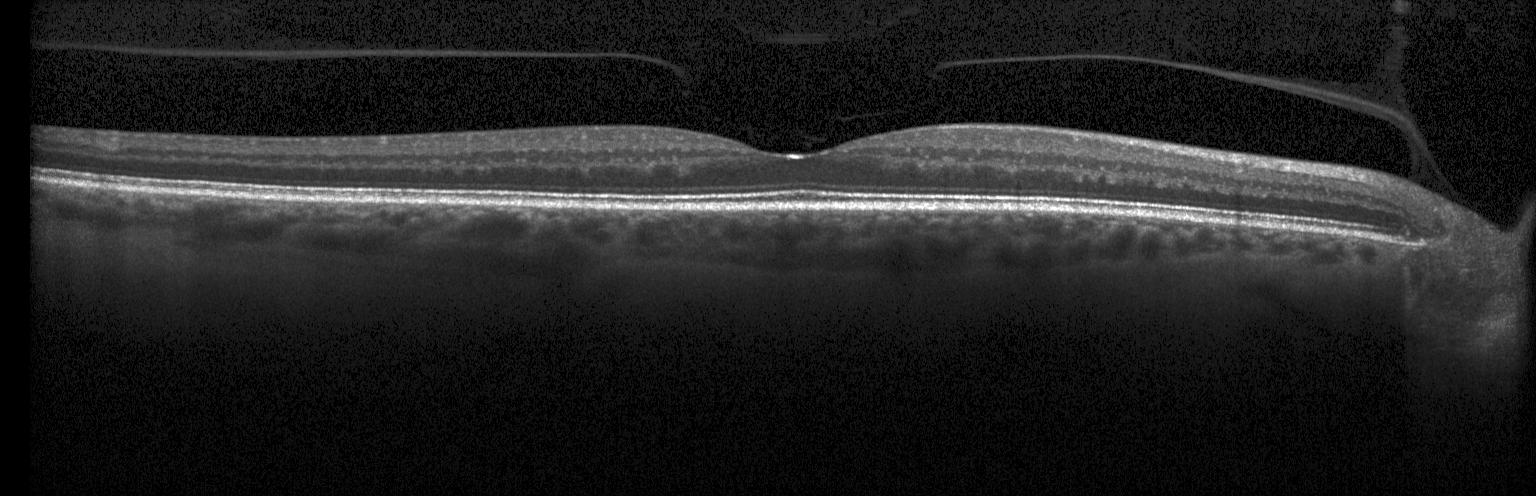 Diagnosis: no evidence of choroidal neovascularization, diabetic macular edema, or drusen.